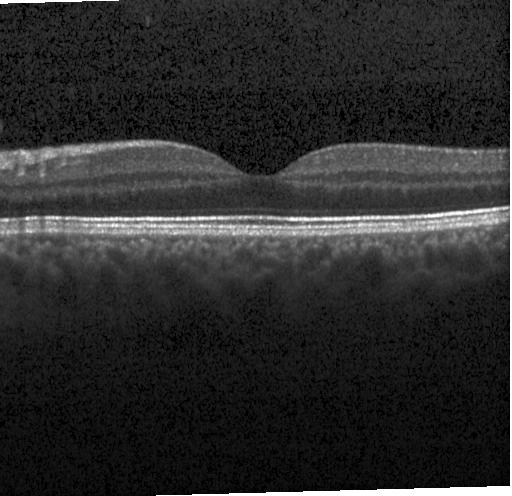

Heidelberg Spectralis · OCT line scan · spectral-domain optical coherence tomography · macular scan
Assessment: no evidence of choroidal neovascularization, diabetic macular edema, or drusen.